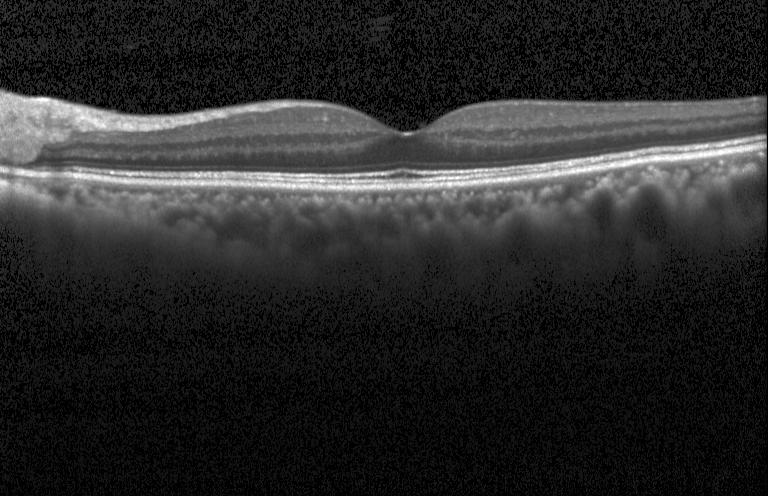

Retinal OCT B-scan, fovea-centered, spectral-domain OCT, acquired on a Heidelberg Spectralis.
Impression: no evidence of choroidal neovascularization, diabetic macular edema, or drusen.